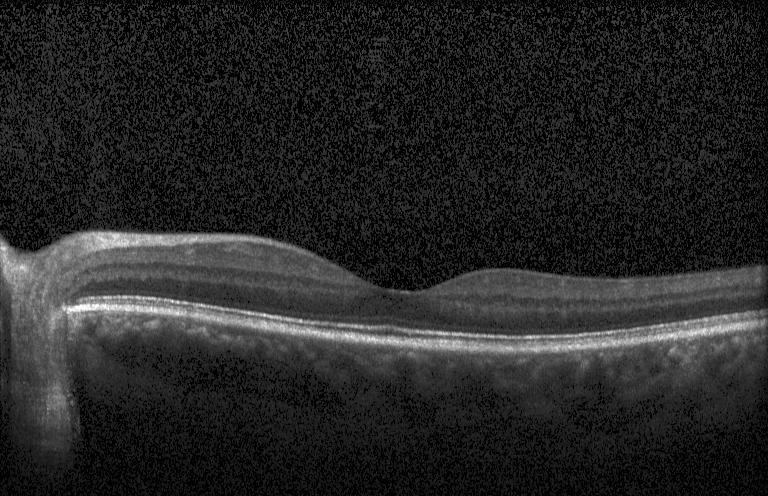

Finding: no CNV, DME, or drusen.